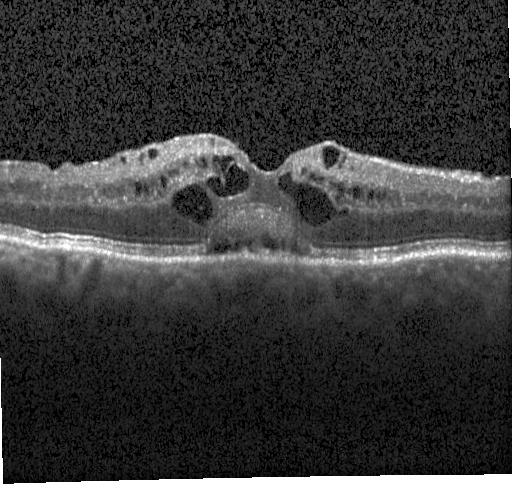 OCT B-scan.
OCT finding: diabetic macular edema (DME).